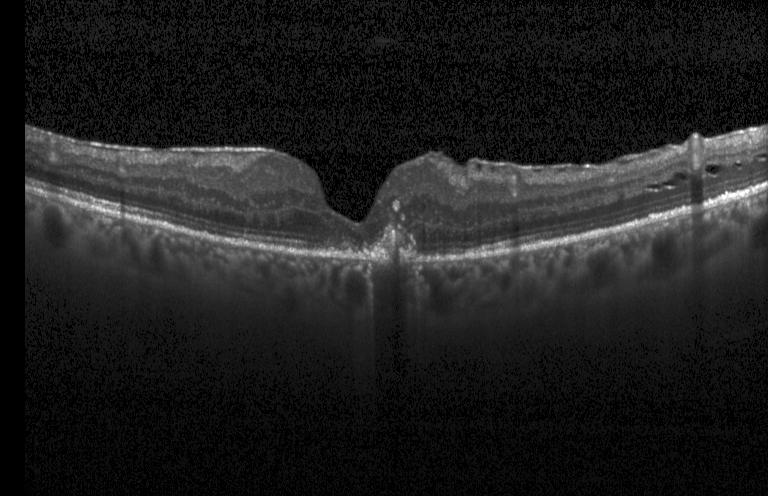 Finding: choroidal neovascularization.